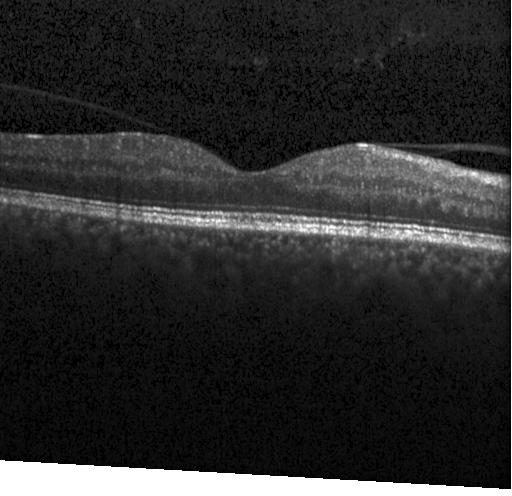

Diagnosis: no CNV, DME, or drusen.